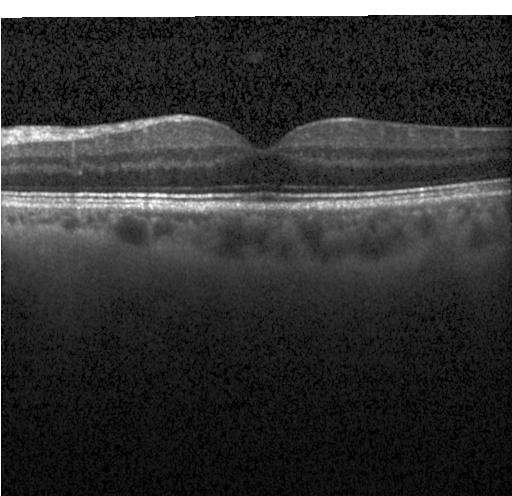
Spectral-domain optical coherence tomography. OCT line scan — Macular OCT: no choroidal neovascularization, no diabetic macular edema, and no drusen.